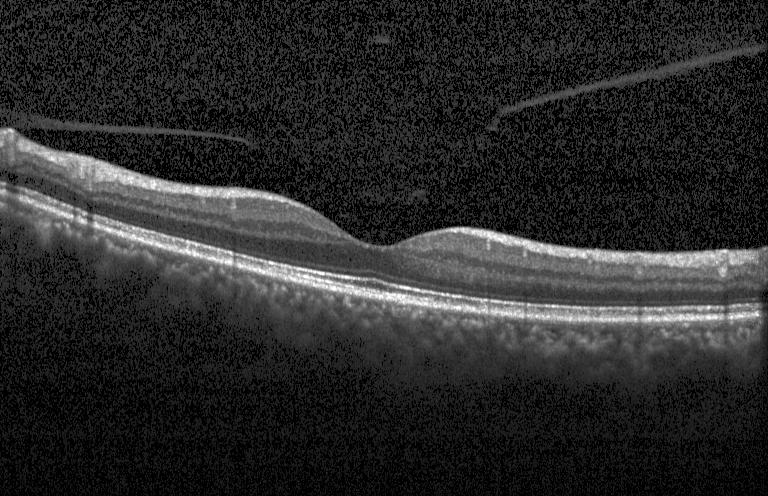 Neither choroidal neovascularization, diabetic macular edema, nor drusen.